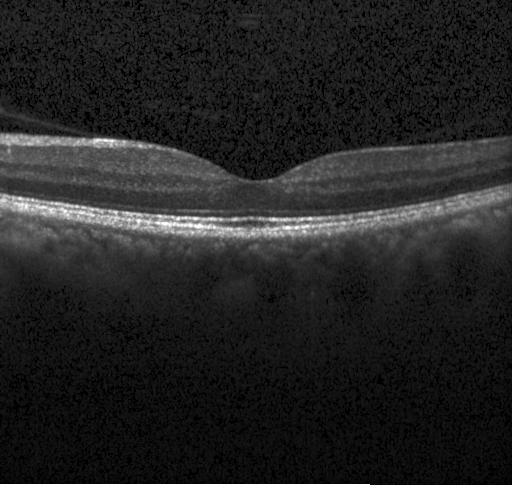

Spectral-domain OCT; instrument: Heidelberg Spectralis; optical coherence tomography scan. Diagnosis: no evidence of choroidal neovascularization, diabetic macular edema, or drusen.